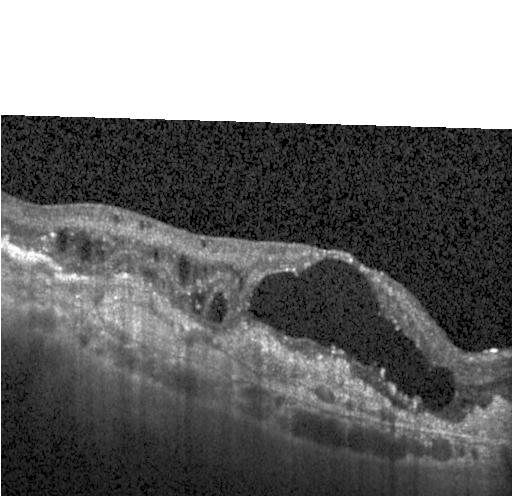
OCT B-scan showing choroidal neovascularization (CNV).